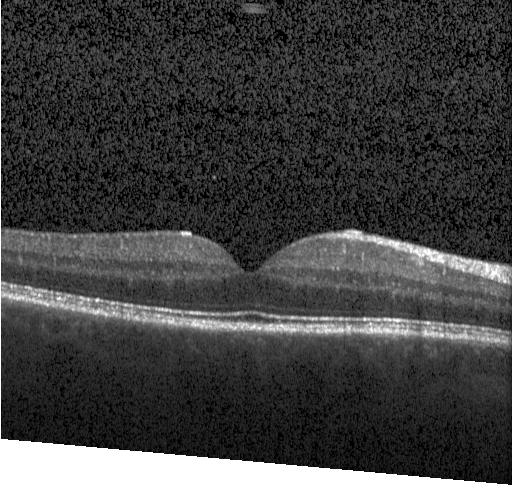
Retinal OCT B-scan. Instrument: Heidelberg Spectralis — This B-scan demonstrates no choroidal neovascularization, diabetic macular edema, or drusen.